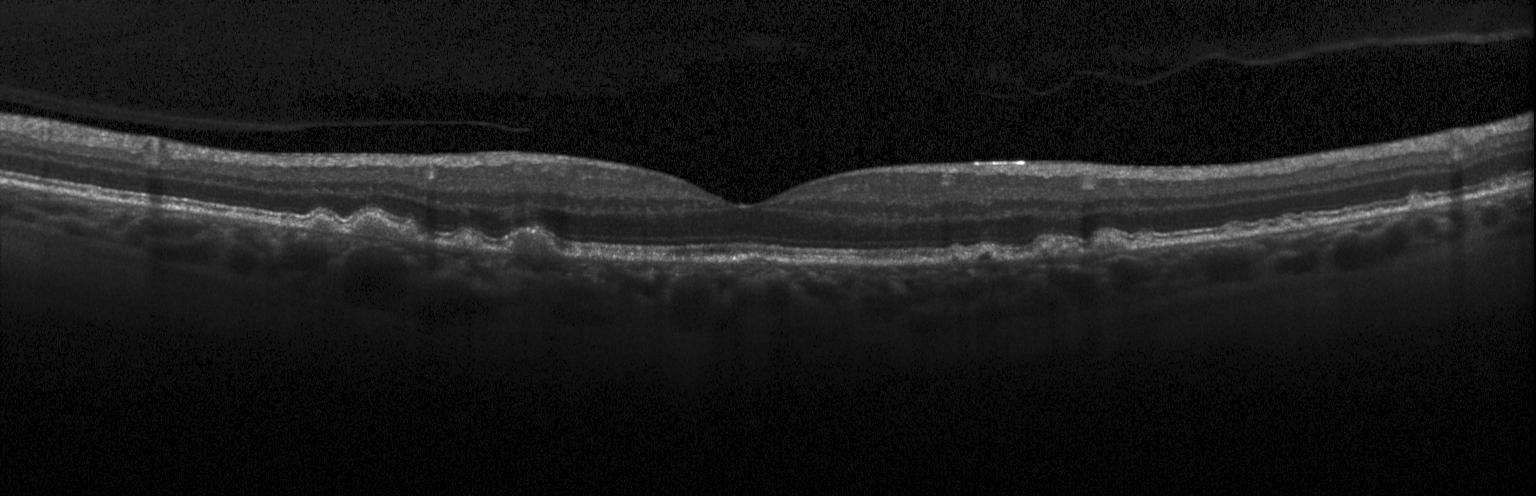 Heidelberg Spectralis OCT system · retinal OCT B-scan — Finding: drusen.